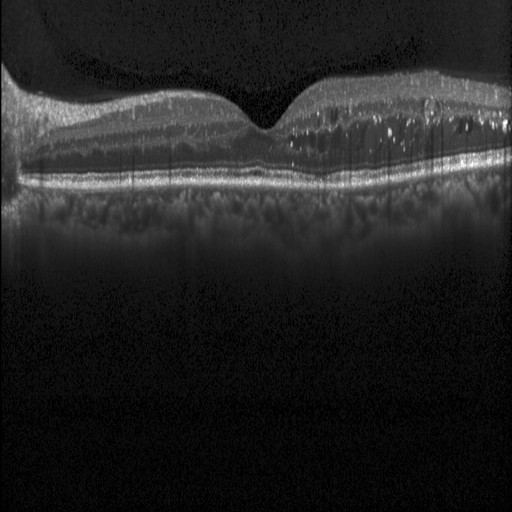

OCT line scan; macular scan — OCT finding: diabetic macular edema.